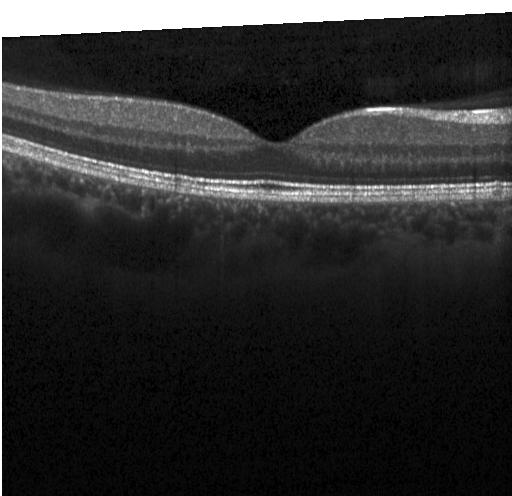

OCT scan showing no choroidal neovascularization, diabetic macular edema, or drusen.